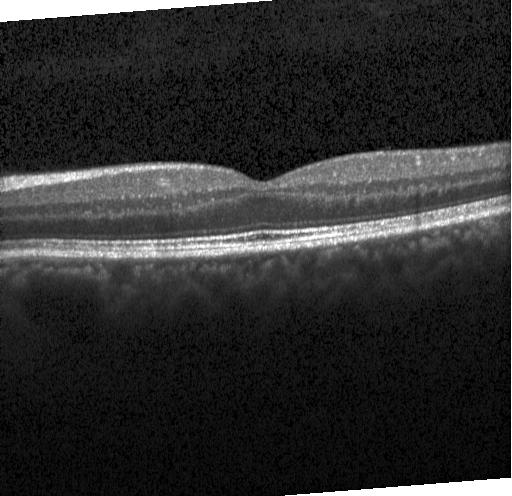

Impression: no evidence of choroidal neovascularization, diabetic macular edema, or drusen.